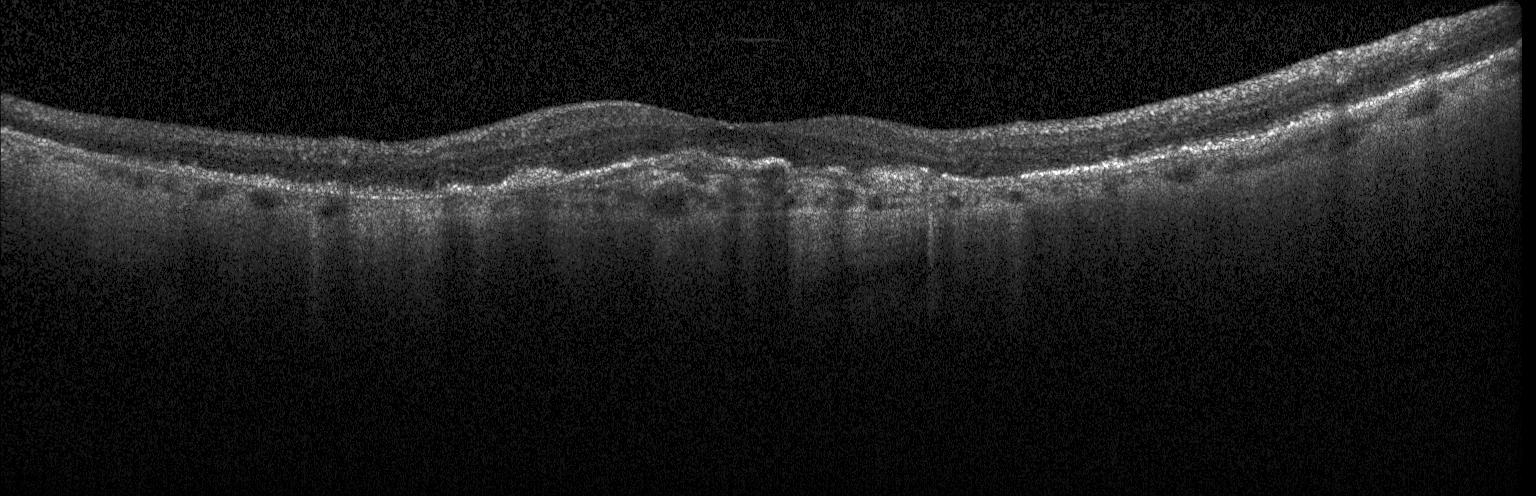 OCT B-scan
OCT finding: a choroidal neovascular membrane.